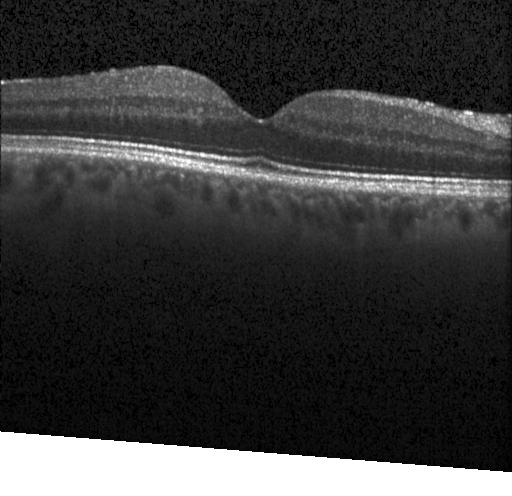
Assessment: no evidence of choroidal neovascularization, diabetic macular edema, or drusen.